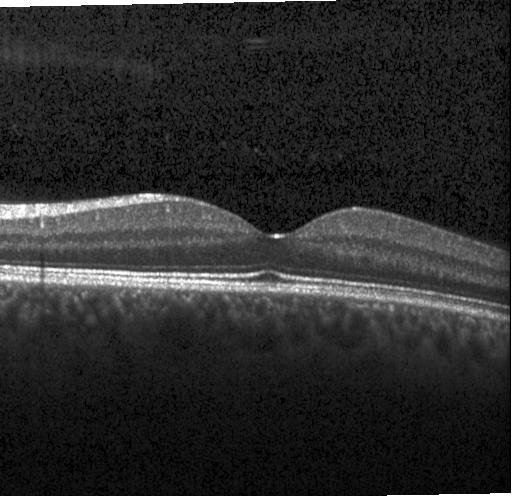
Retinal OCT B-scan
Finding: no choroidal neovascularization, diabetic macular edema, or drusen.